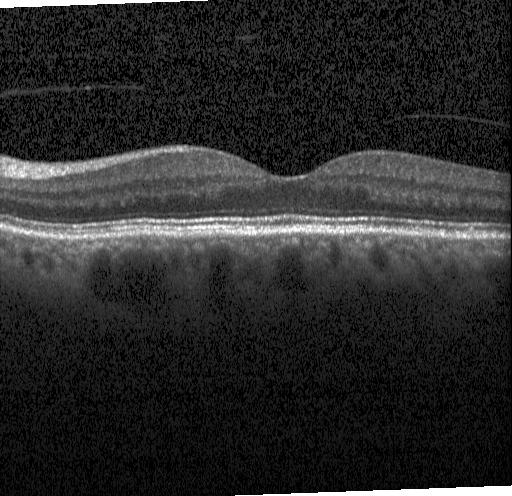
Retinal OCT cross-section showing no choroidal neovascularization, diabetic macular edema, or drusen.